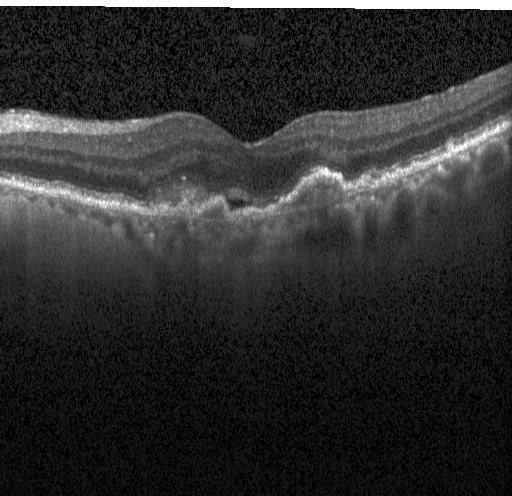
OCT line scan. Through the macula. Spectral-domain OCT. Heidelberg Spectralis OCT system. Impression: choroidal neovascularization (CNV).